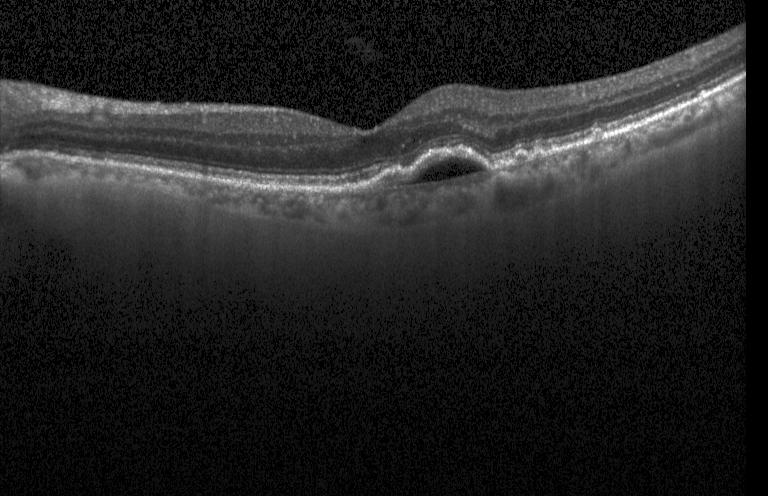 OCT line scan. Heidelberg Spectralis.
OCT finding: choroidal neovascularization (CNV).